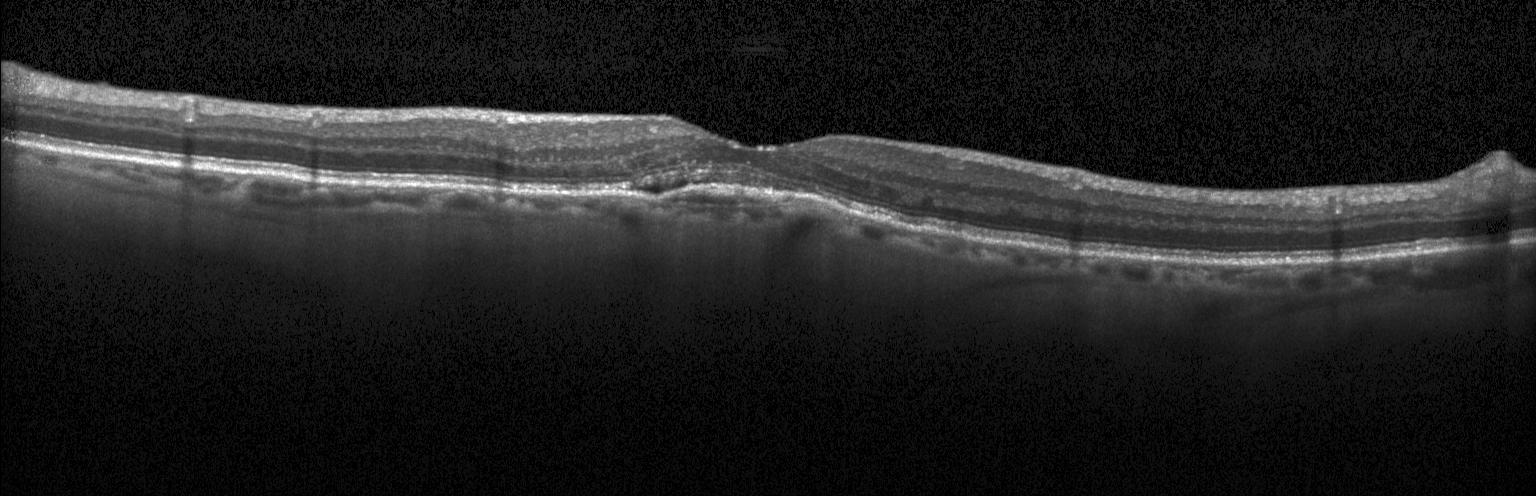 Spectral-domain OCT B-scan: choroidal neovascularization (CNV).